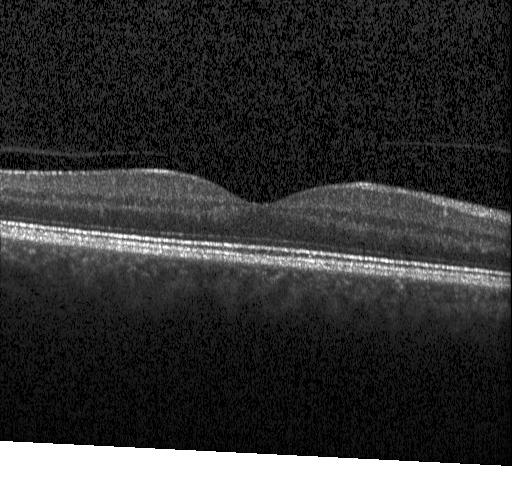
Fovea-centered. SD-OCT. OCT B-scan
Macular OCT: no CNV, DME, or drusen.